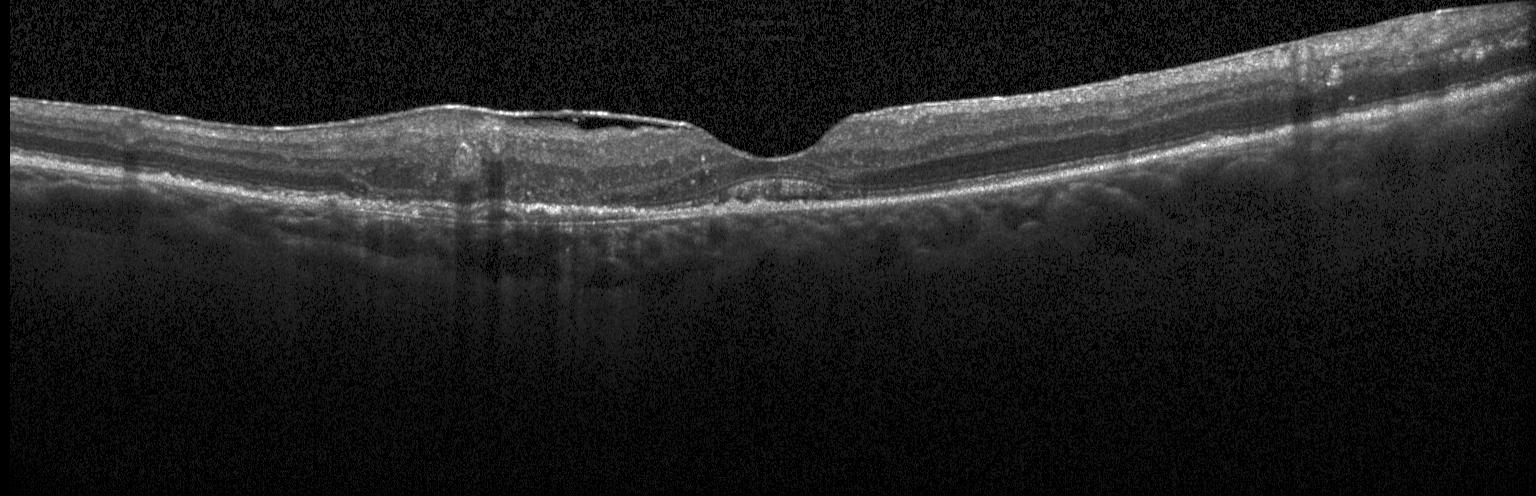

Impression: CNV.